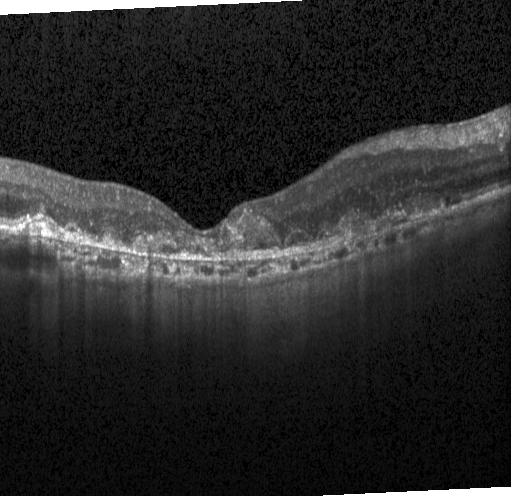 Through the macula · retinal OCT B-scan · Heidelberg Spectralis OCT system
CNV.